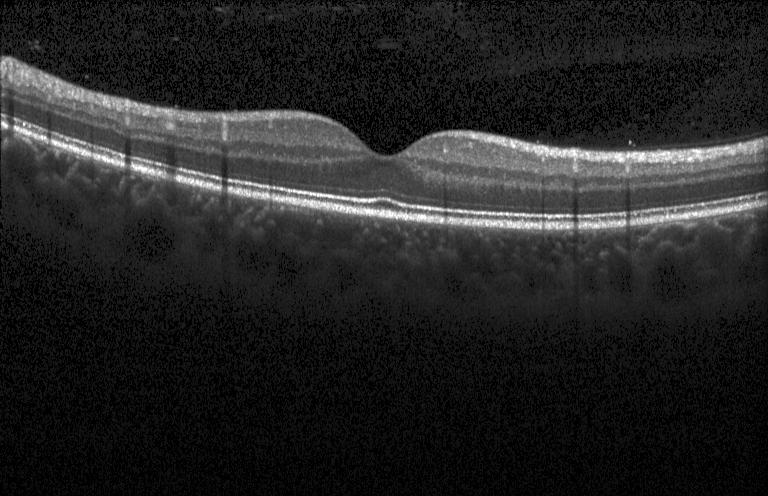

Optical coherence tomography scan
Macular OCT: neither CNV, DME, nor drusen.